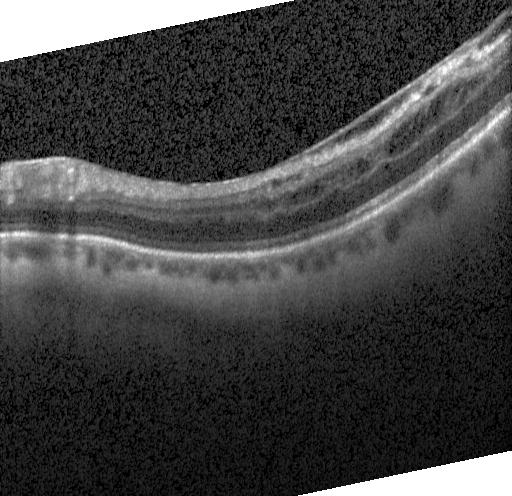

Macular OCT demonstrating diabetic macular edema (DME).